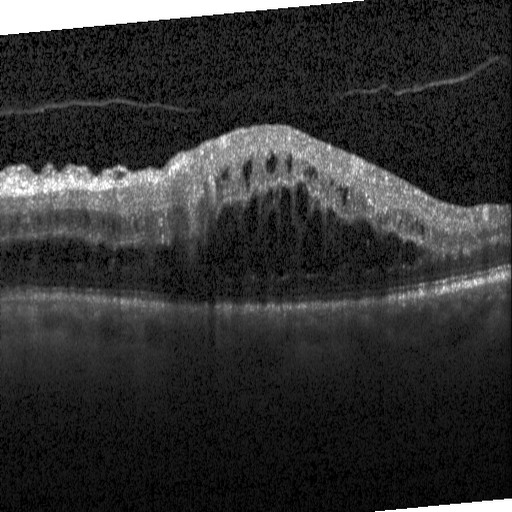 Centered on the fovea. Spectral-domain optical coherence tomography. Retinal OCT cross-section
Impression: diabetic macular edema.